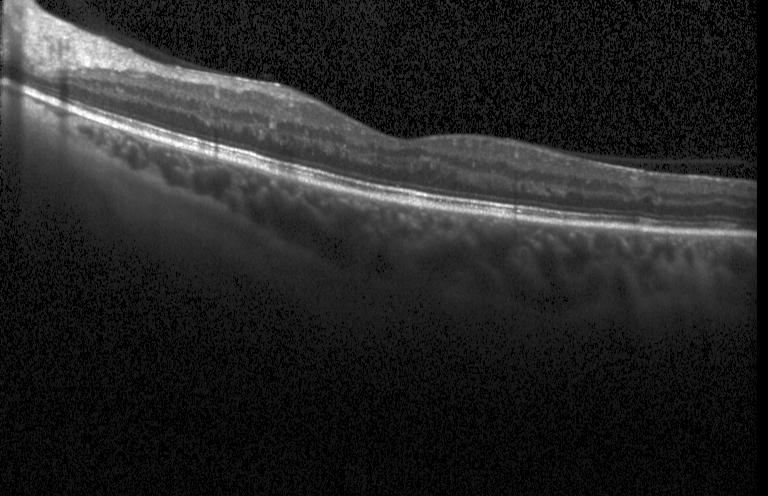
Impression: no evidence of choroidal neovascularization, diabetic macular edema, or drusen.